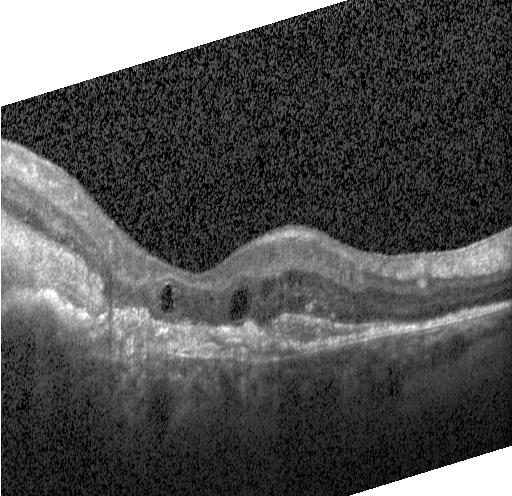

OCT finding: CNV.